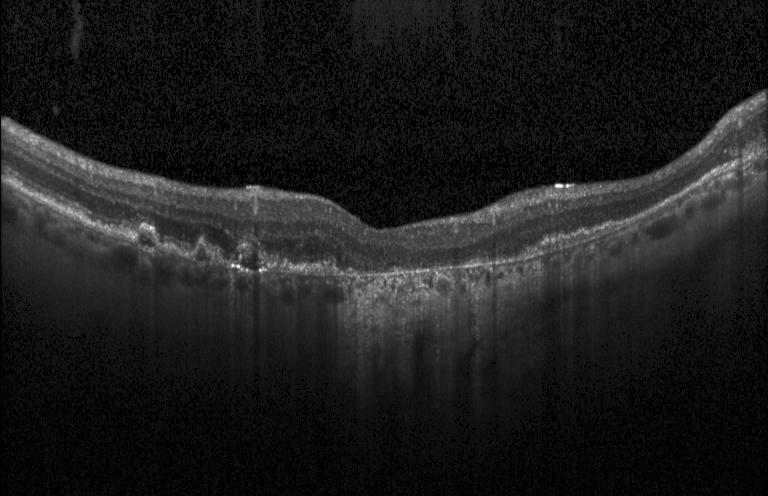
Fovea-centered. Spectral-domain optical coherence tomography. OCT B-scan.
This B-scan demonstrates a choroidal neovascular membrane.